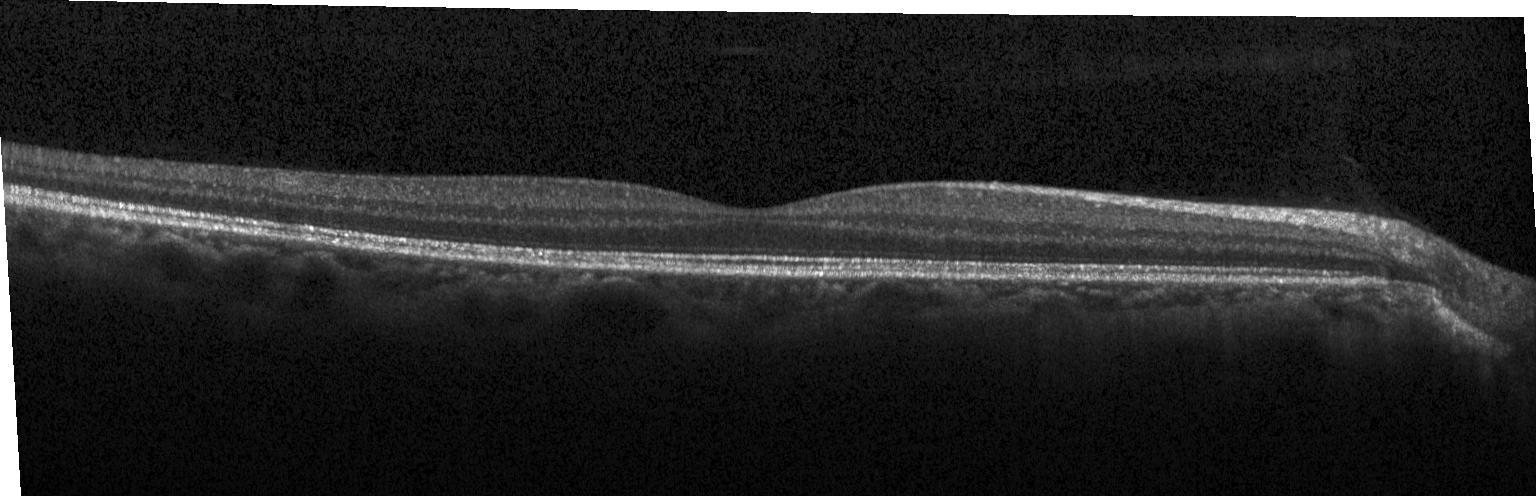

OCT B-scan, spectral-domain optical coherence tomography
Macular OCT: no CNV, no DME, and no drusen.